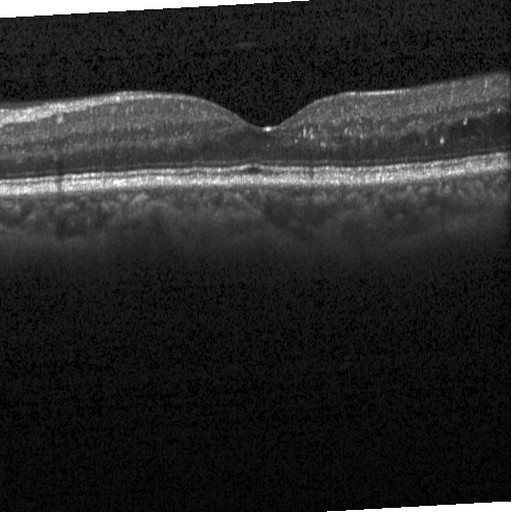

Heidelberg Spectralis OCT system. Retinal OCT B-scan. SD-OCT
Impression: diabetic macular edema (DME).